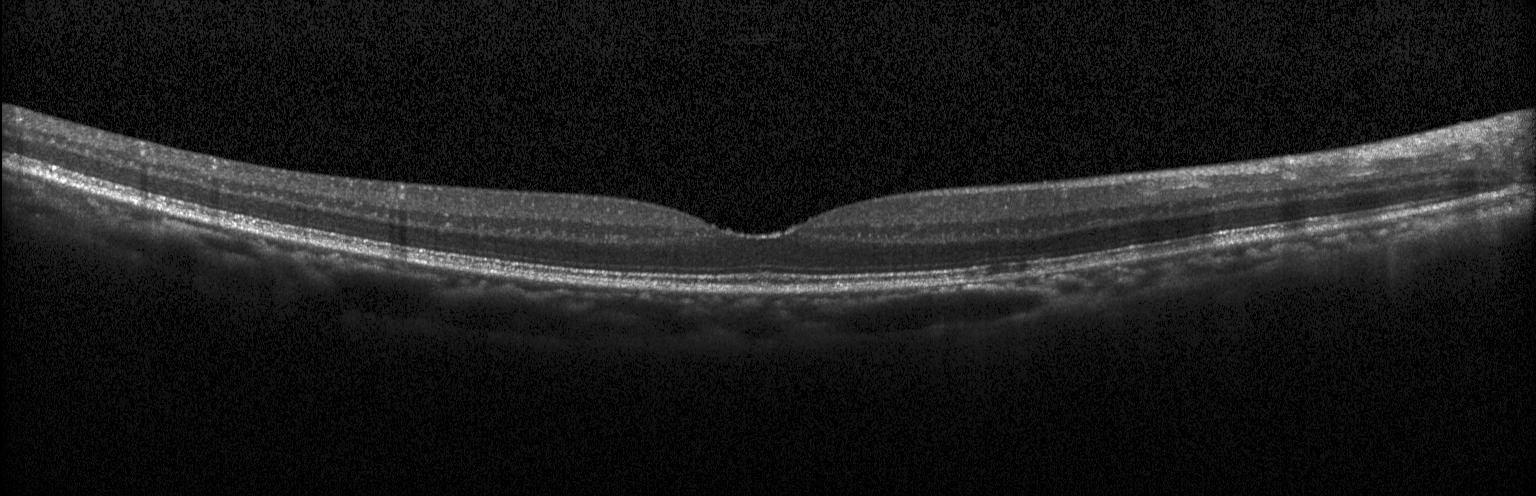 Spectral-domain OCT. Optical coherence tomography B-scan. Assessment: no choroidal neovascularization, no diabetic macular edema, and no drusen.